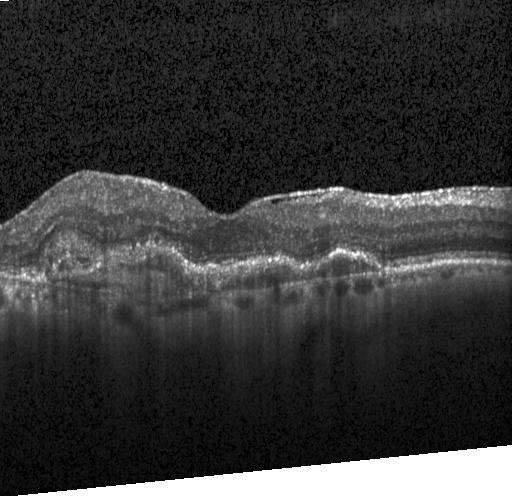

OCT B-scan showing a choroidal neovascular membrane.